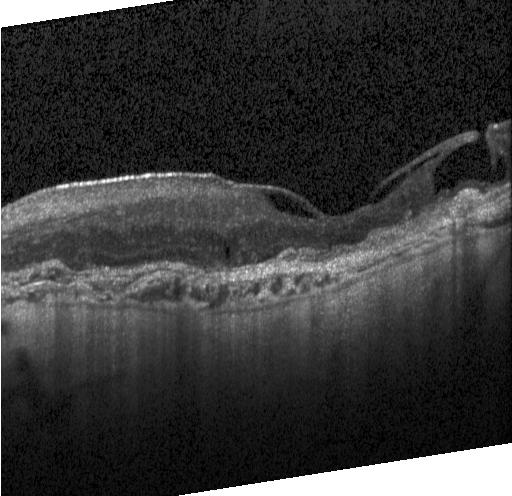

Finding: a choroidal neovascular membrane.